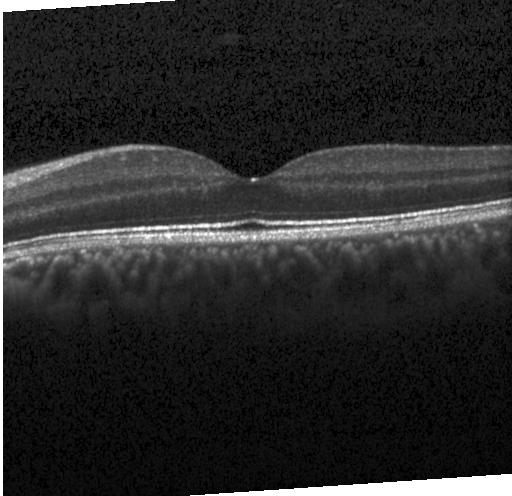
Spectral-domain OCT B-scan: no choroidal neovascularization, no diabetic macular edema, and no drusen.